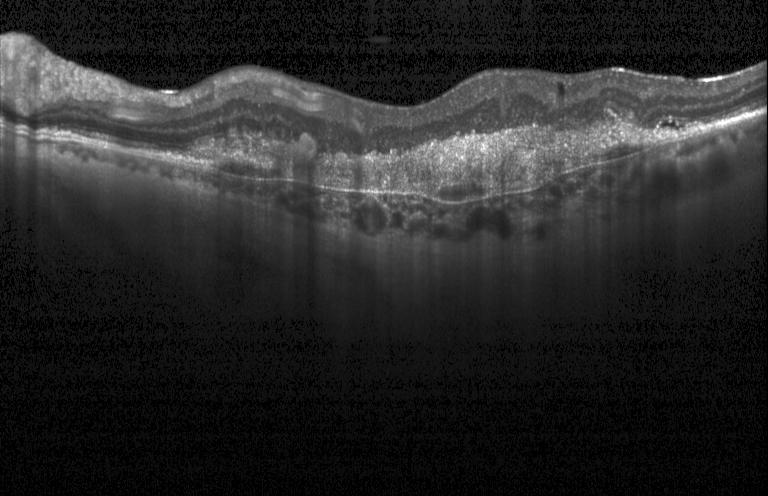

CNV.